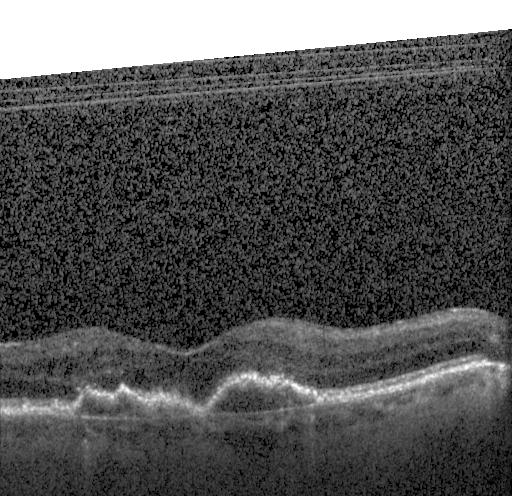
OCT line scan; through the macula
Impression: choroidal neovascularization.